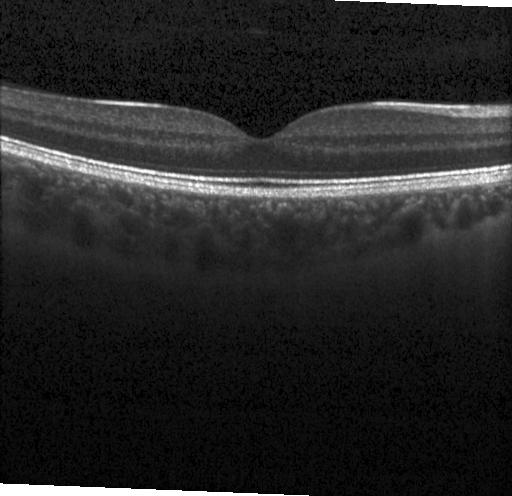 This B-scan demonstrates neither choroidal neovascularization, diabetic macular edema, nor drusen.